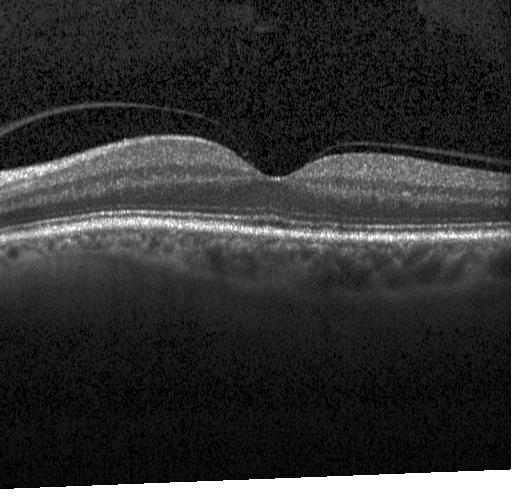 Optical coherence tomography scan.
Impression: no evidence of CNV, DME, or drusen.